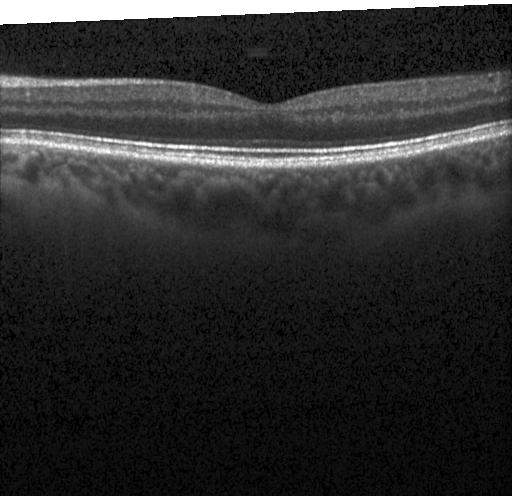
Diagnosis: no choroidal neovascularization, diabetic macular edema, or drusen.